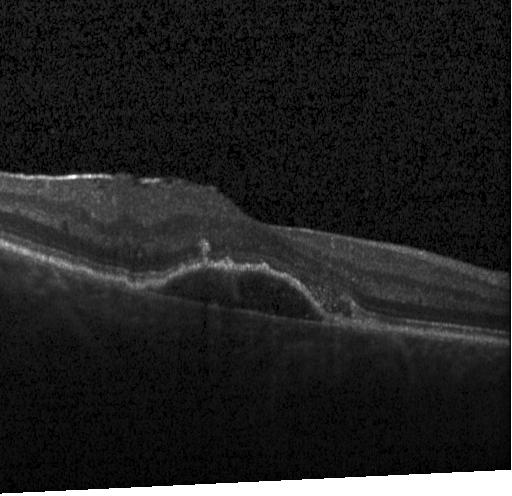
Retinal OCT cross-section showing a choroidal neovascular membrane.